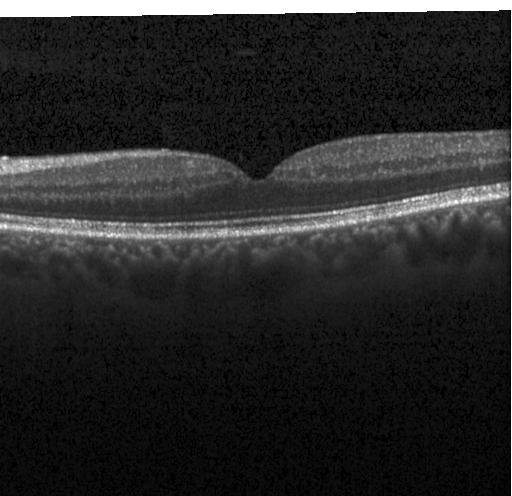 Optical coherence tomography scan
Impression: neither choroidal neovascularization, diabetic macular edema, nor drusen.